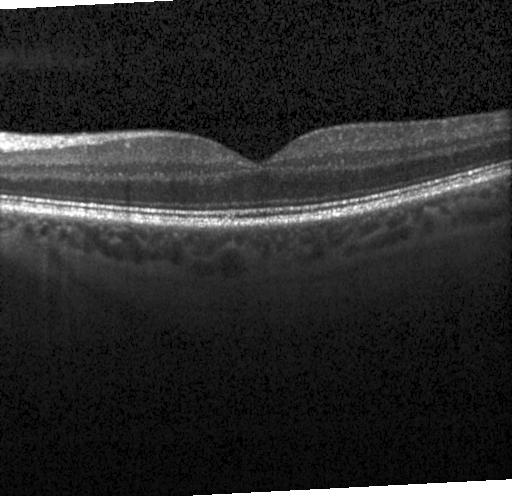
OCT B-scan, SD-OCT, macular scan, Heidelberg Spectralis OCT system. Finding: no choroidal neovascularization, no diabetic macular edema, and no drusen.